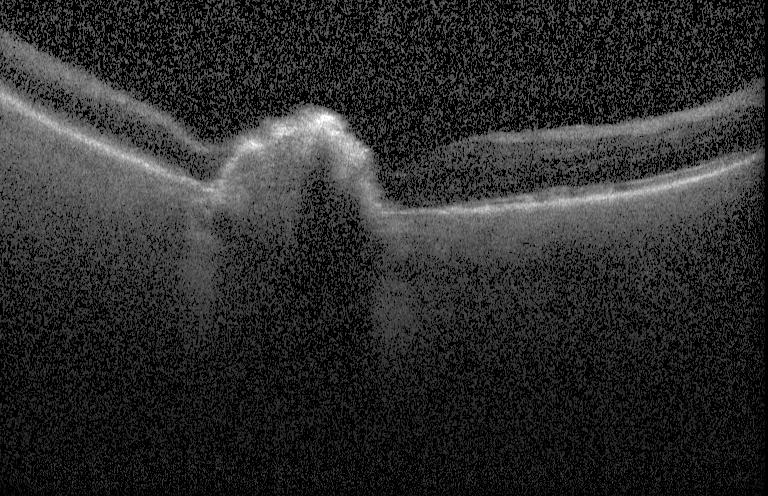

Optical coherence tomography scan.
Diagnosis: CNV.